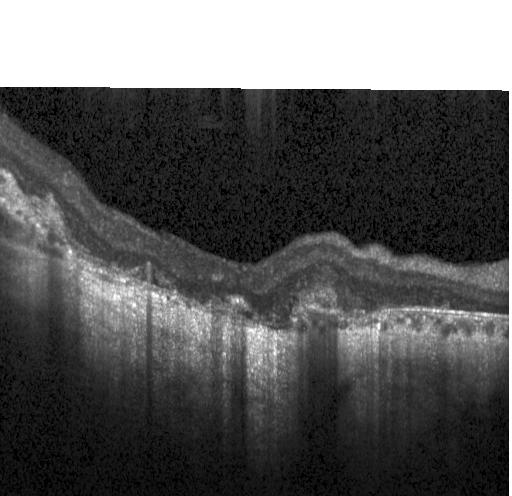 Optical coherence tomography scan, spectral-domain OCT, through the macula. This B-scan demonstrates a choroidal neovascular membrane.